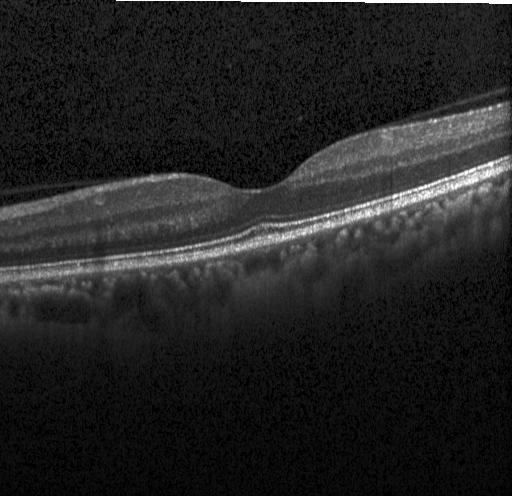
Horizontal scan through the fovea · spectral-domain optical coherence tomography · Heidelberg Spectralis · retinal OCT cross-section.
OCT finding: no CNV, no DME, and no drusen.